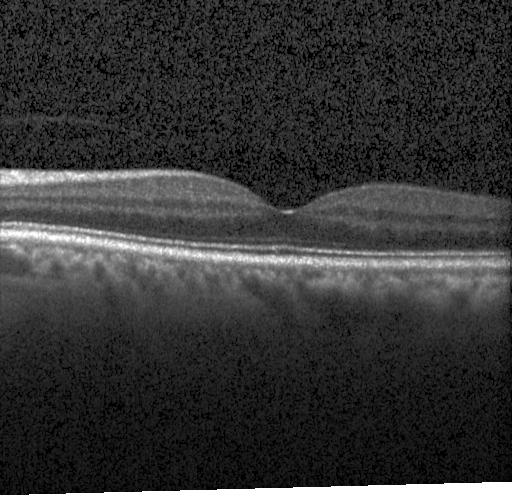

Impression: neither CNV, DME, nor drusen.